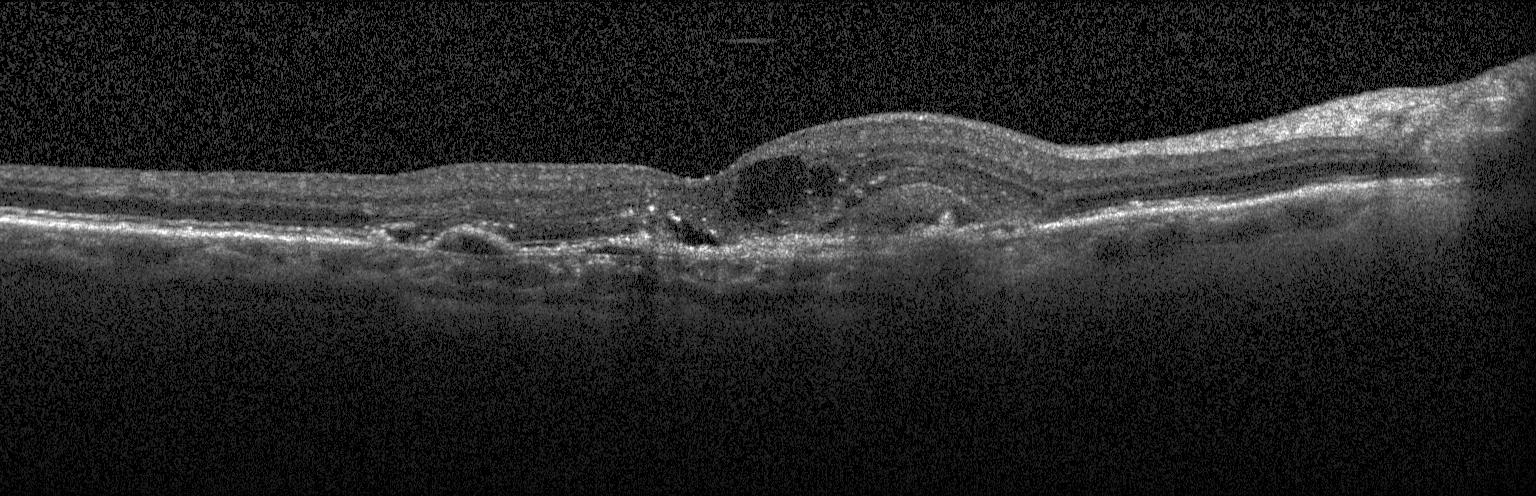
Spectral-domain OCT · retinal OCT B-scan · acquired on a Heidelberg Spectralis · macular scan — OCT finding: a choroidal neovascular membrane.